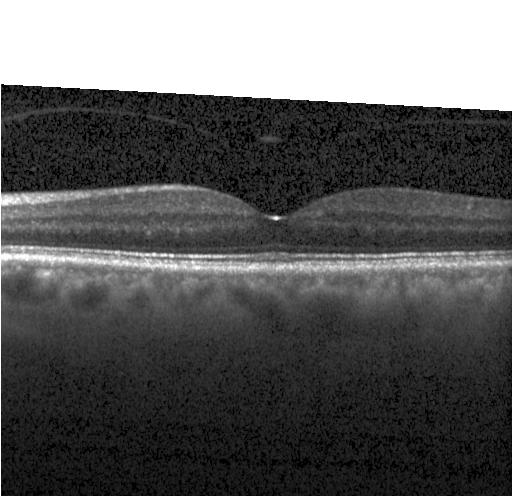
Optical coherence tomography scan. Finding: neither choroidal neovascularization, diabetic macular edema, nor drusen.